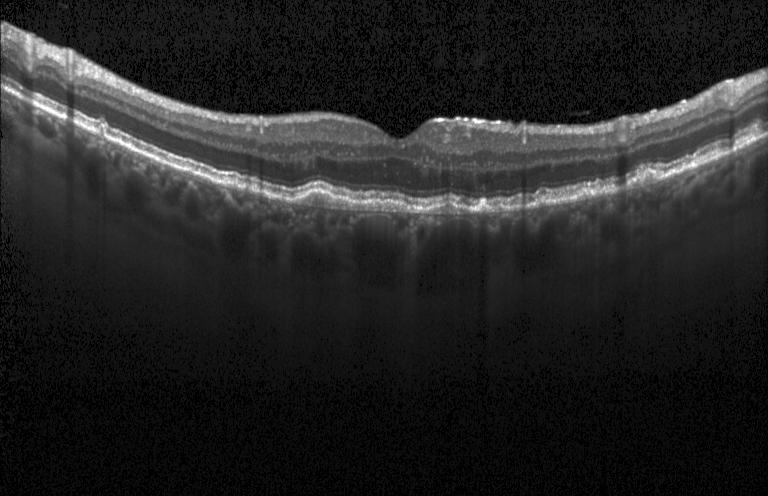
Spectral-domain optical coherence tomography; OCT line scan; Heidelberg Spectralis; fovea-centered.
A choroidal neovascular membrane.